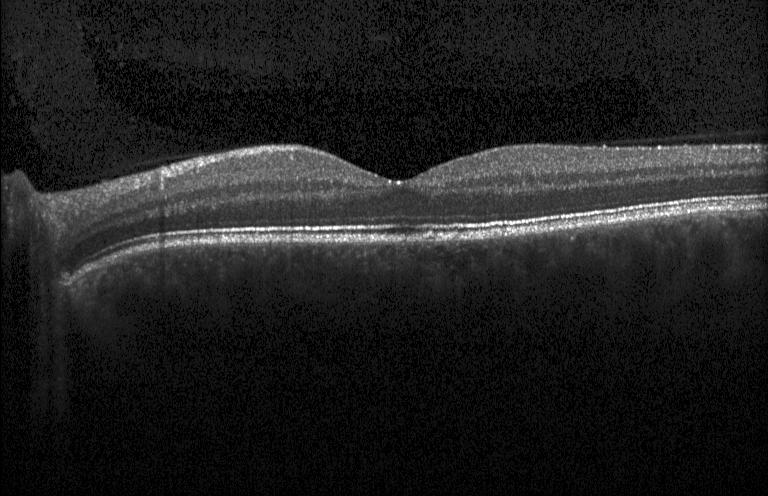
Optical coherence tomography scan. Macular OCT: no choroidal neovascularization, no diabetic macular edema, and no drusen.